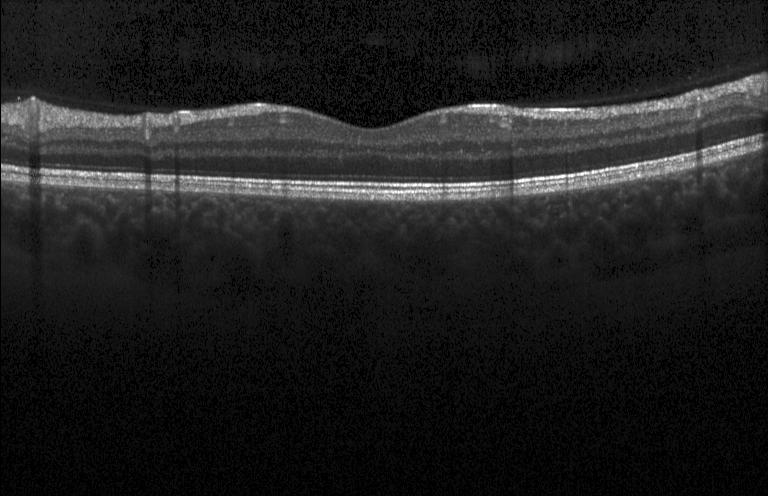 Assessment: no CNV, no DME, and no drusen.